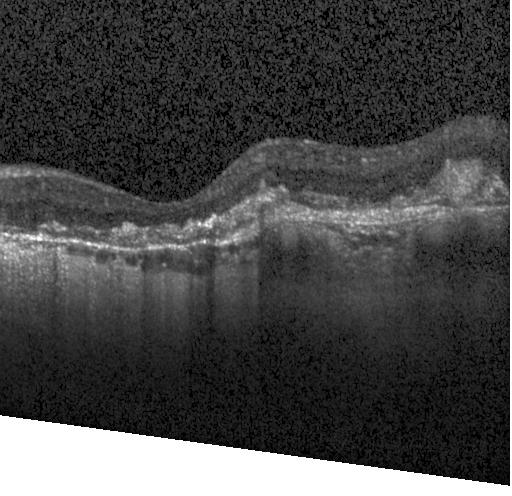
Acquired on a Heidelberg Spectralis. Horizontal scan through the fovea. Retinal OCT cross-section. Spectral-domain OCT.
Finding: choroidal neovascularization.